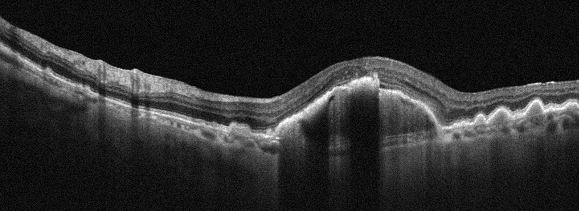 Optovue Avanti RTVue XR. Retinal OCT cross-section. The scan shows age-related macular degeneration.